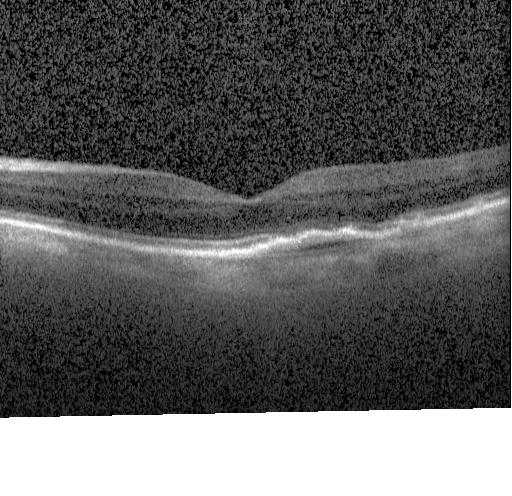

Instrument: Heidelberg Spectralis; fovea-centered; optical coherence tomography B-scan; spectral-domain optical coherence tomography
A choroidal neovascular membrane.